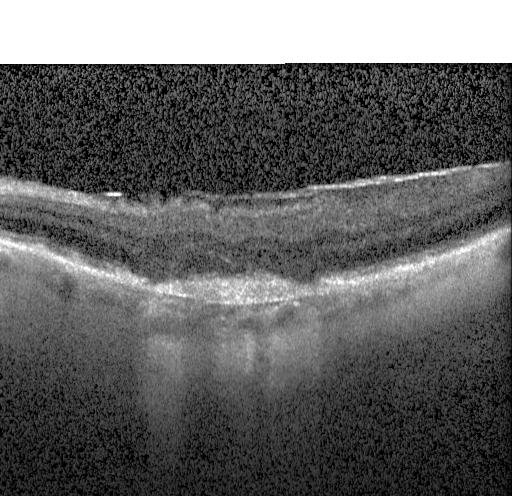
Retinal OCT B-scan; macular scan. Macular OCT: CNV.